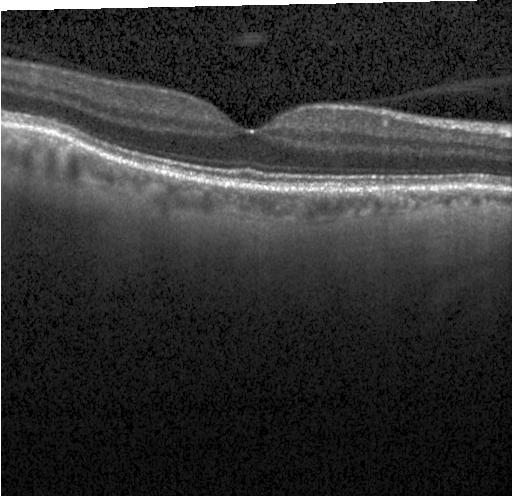 OCT line scan · spectral-domain optical coherence tomography · acquired on a Heidelberg Spectralis · through the macula — No choroidal neovascularization, diabetic macular edema, or drusen.